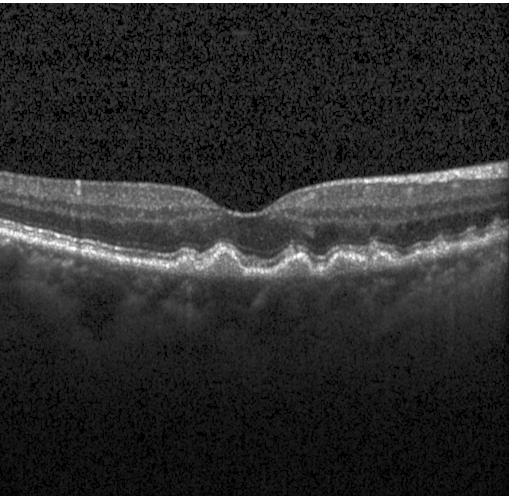
SD-OCT. Optical coherence tomography B-scan. Horizontal scan through the fovea — Dx: multiple drusen.